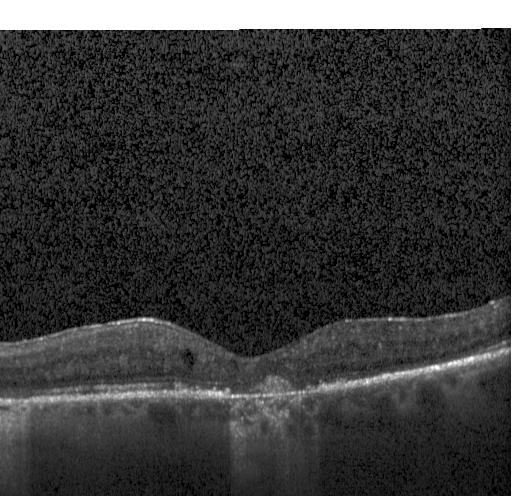

Macular OCT: choroidal neovascularization (CNV).